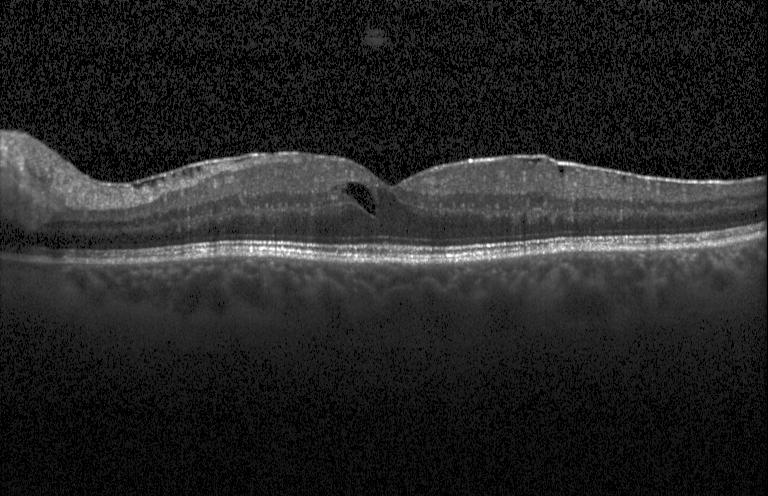
Macular OCT demonstrating diabetic macular edema (DME).